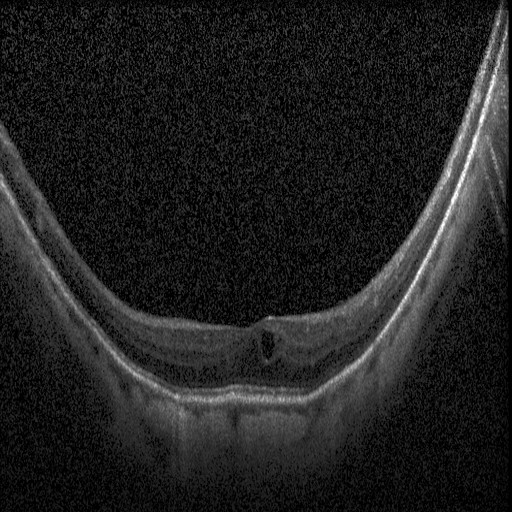 Optical coherence tomography scan · spectral-domain optical coherence tomography · acquired on a Heidelberg Spectralis · fovea-centered — Finding: diabetic macular edema (DME).